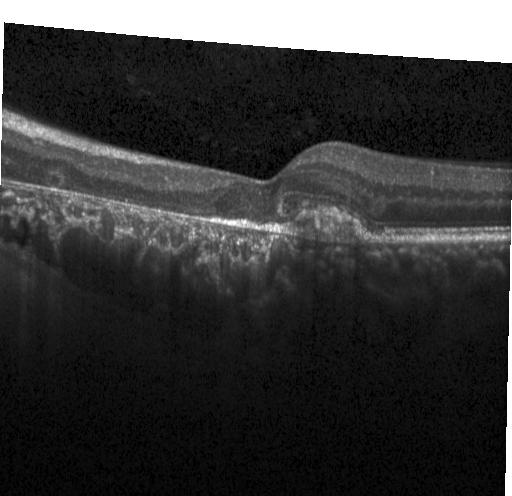
Assessment: CNV.